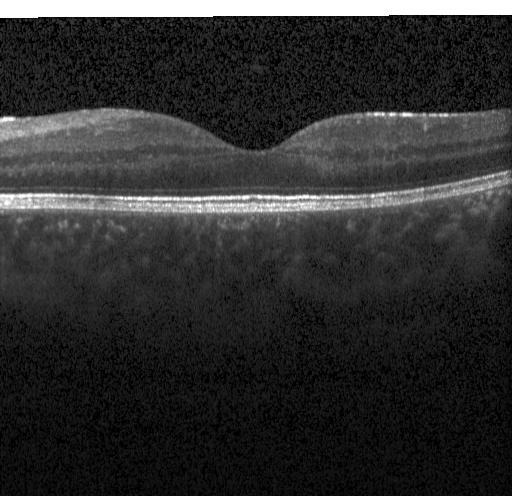
Retinal OCT B-scan. Macular OCT: neither choroidal neovascularization, diabetic macular edema, nor drusen.